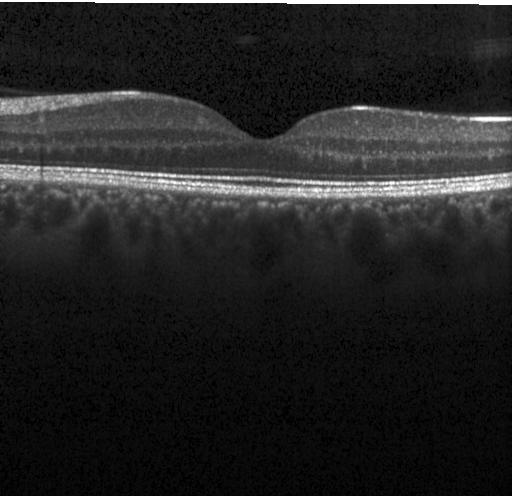 SD-OCT, macular scan, retinal OCT cross-section
Diagnosis: no choroidal neovascularization, diabetic macular edema, or drusen.